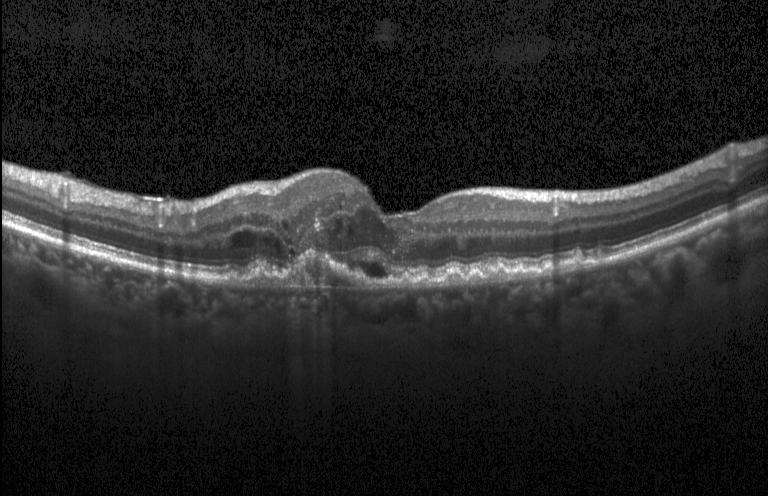

Impression: a choroidal neovascular membrane.